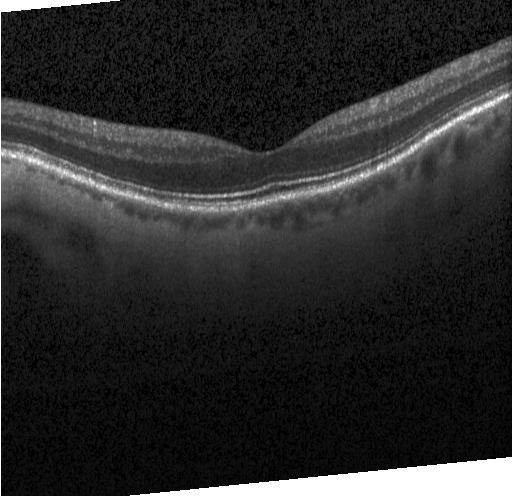 OCT finding: neither CNV, DME, nor drusen.